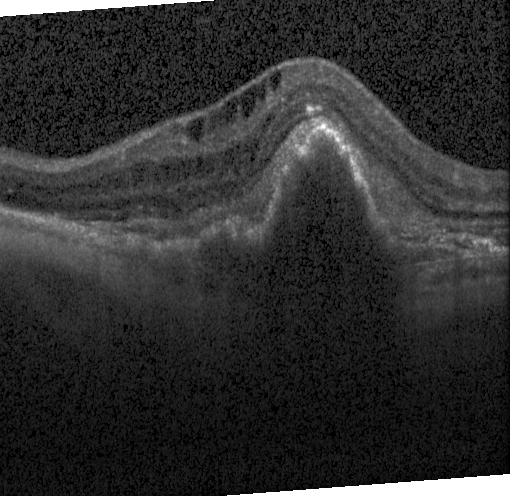
SD-OCT, optical coherence tomography scan, macular scan, instrument: Heidelberg Spectralis — Finding: a choroidal neovascular membrane.